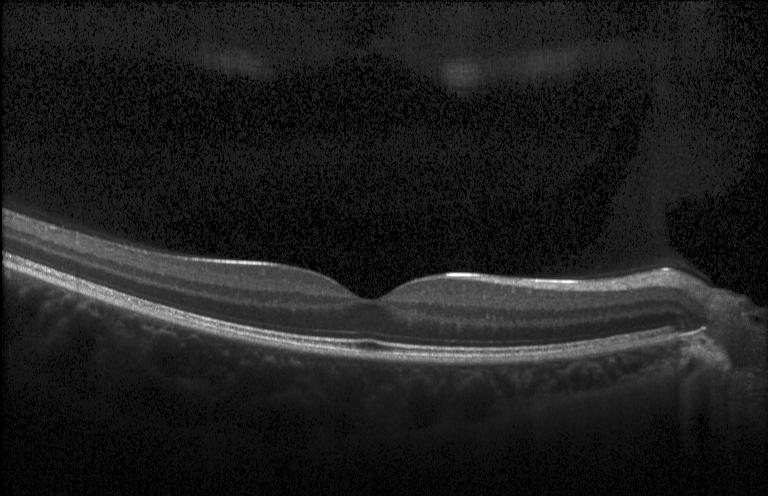

Retinal OCT cross-section; Heidelberg Spectralis — Assessment: no choroidal neovascularization, diabetic macular edema, or drusen.